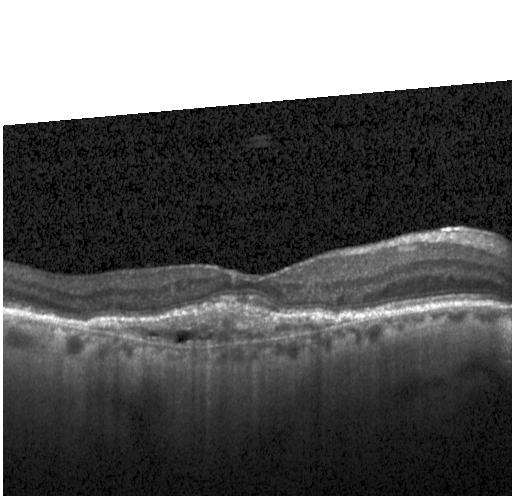
Optical coherence tomography B-scan.
Assessment: choroidal neovascularization (CNV).